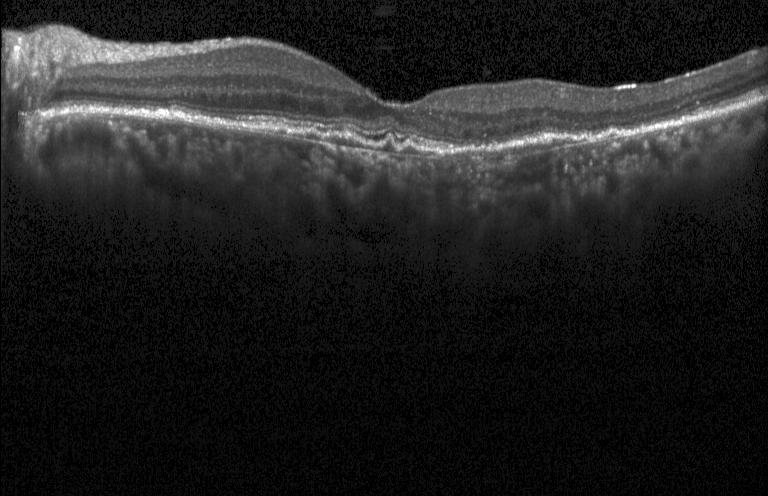 OCT finding: CNV.